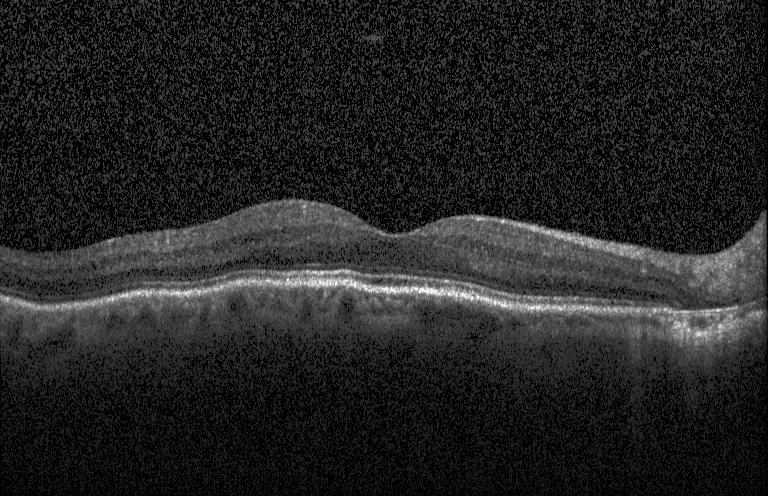

OCT B-scan showing no choroidal neovascularization, no diabetic macular edema, and no drusen.